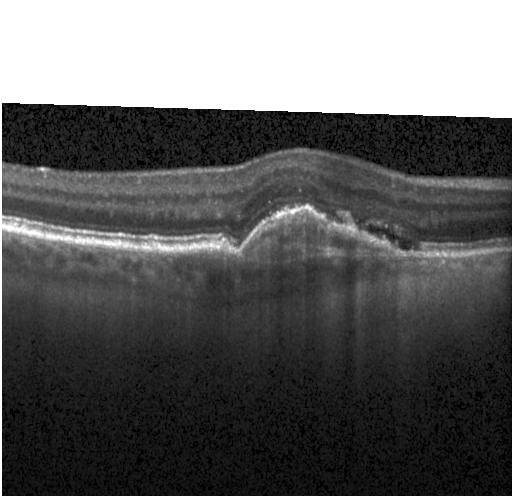

SD-OCT, macular scan, Heidelberg Spectralis, OCT B-scan. Impression: a choroidal neovascular membrane.